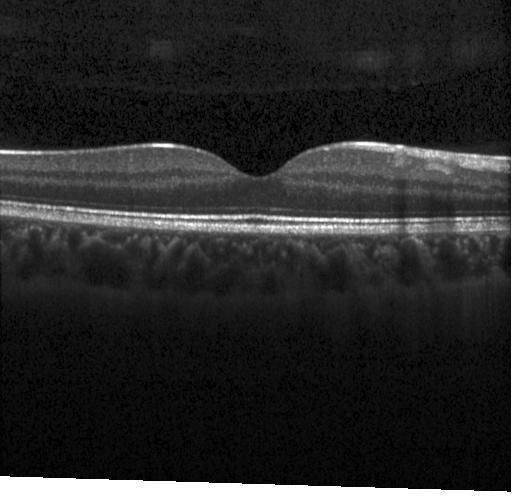 OCT B-scan. Macular OCT: no CNV, DME, or drusen.